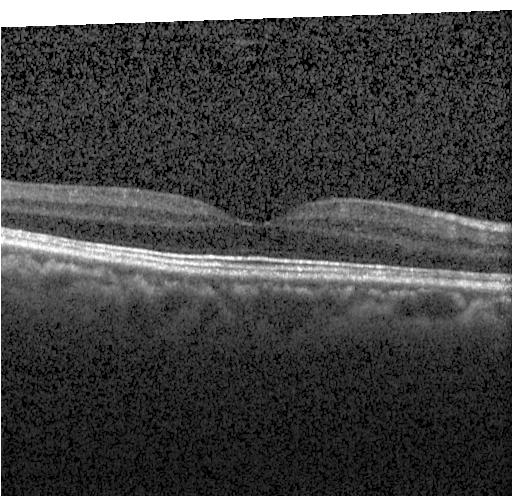 No choroidal neovascularization, no diabetic macular edema, and no drusen.